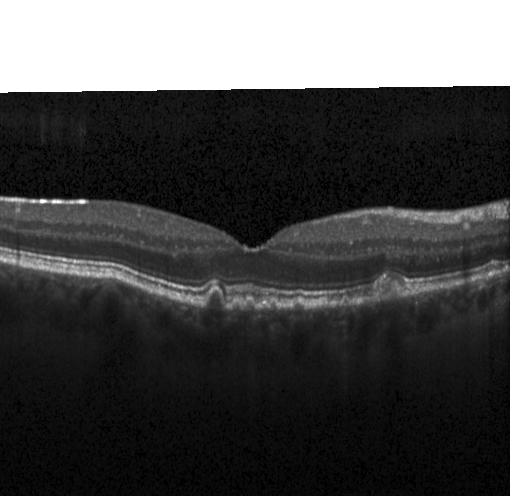
Retinal OCT cross-section · through the macula · Heidelberg Spectralis OCT system · SD-OCT — Sub-RPE drusenoid deposits.